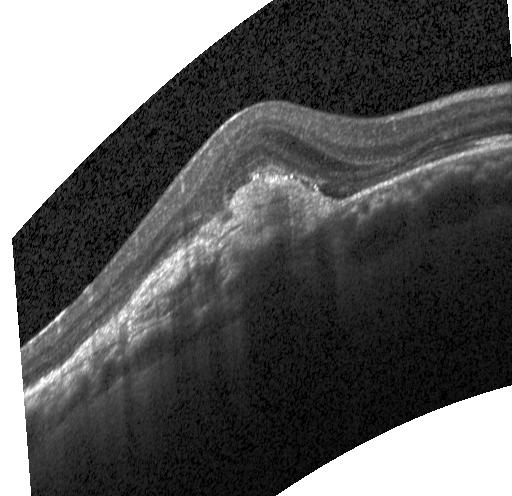

Retinal OCT cross-section showing a choroidal neovascular membrane.